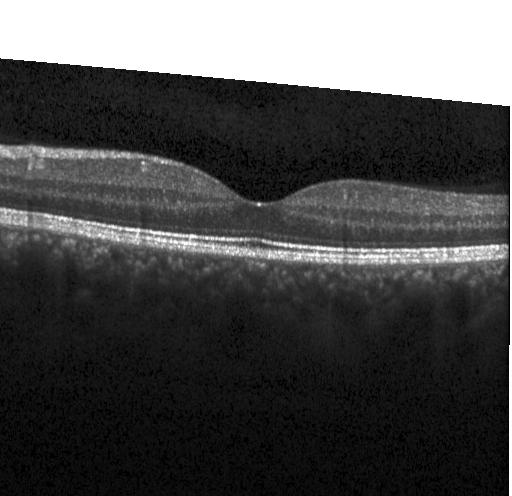 Optical coherence tomography B-scan
Impression: no choroidal neovascularization, no diabetic macular edema, and no drusen.